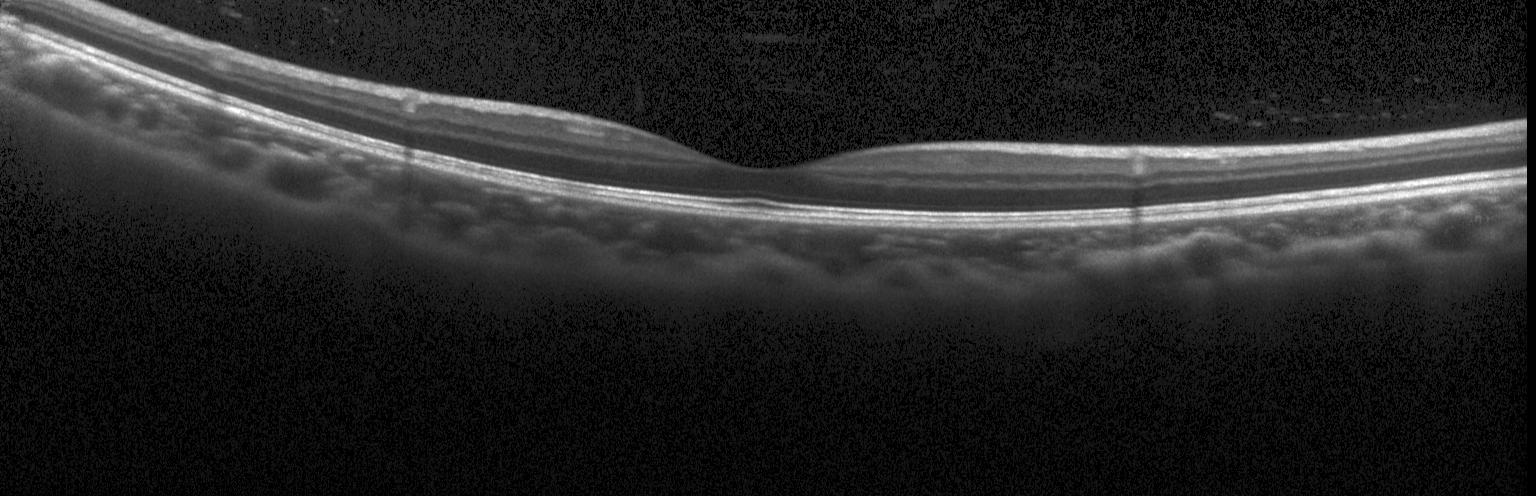
Acquired on a Heidelberg Spectralis, OCT line scan. Assessment: neither CNV, DME, nor drusen.